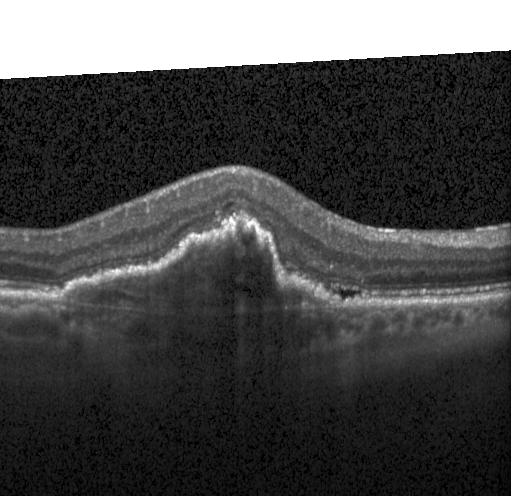

Spectral-domain optical coherence tomography. Heidelberg Spectralis OCT system. Horizontal scan through the fovea. Retinal OCT cross-section. Diagnosis: choroidal neovascularization (CNV).